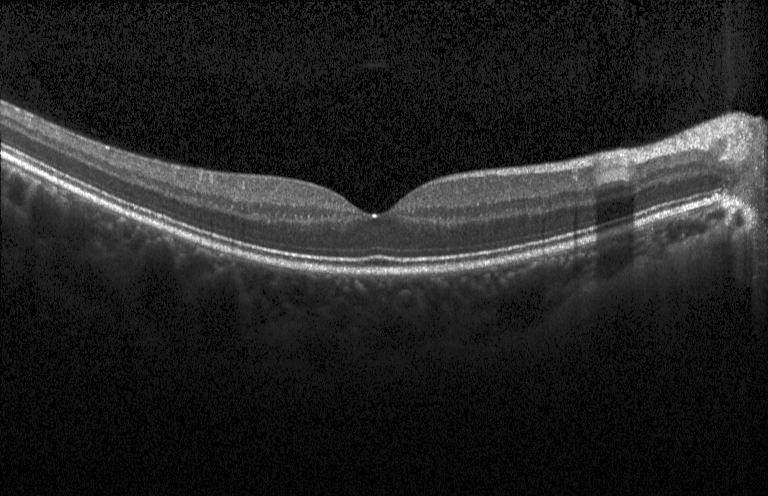 OCT line scan · spectral-domain optical coherence tomography · macular scan — The scan shows no CNV, DME, or drusen.